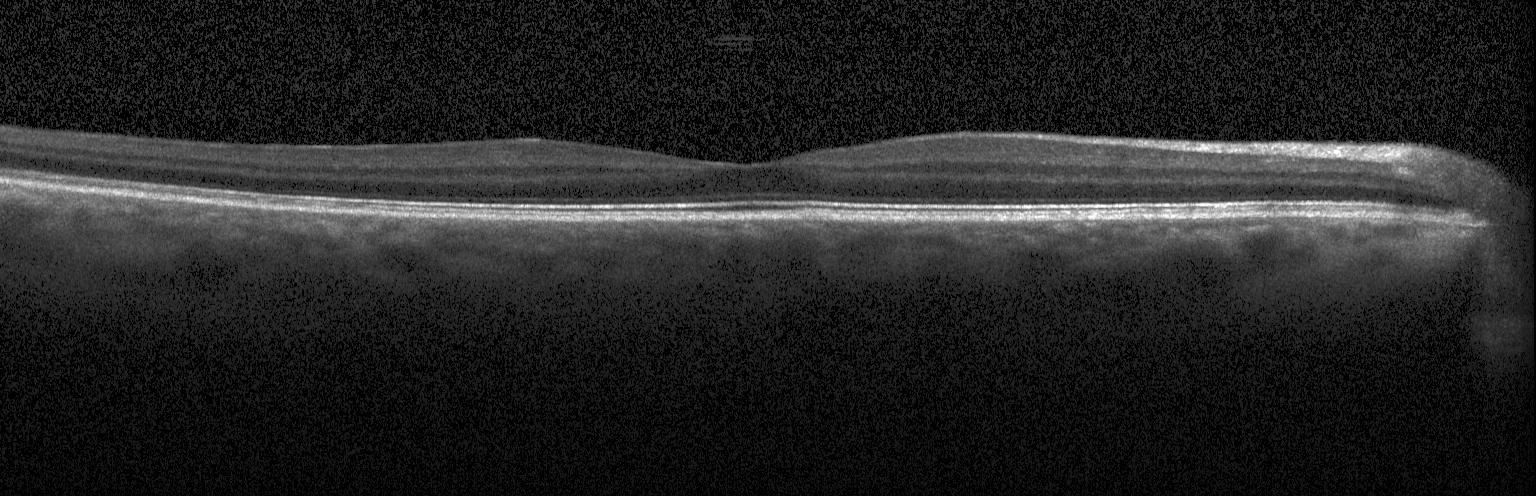
The scan shows neither choroidal neovascularization, diabetic macular edema, nor drusen.